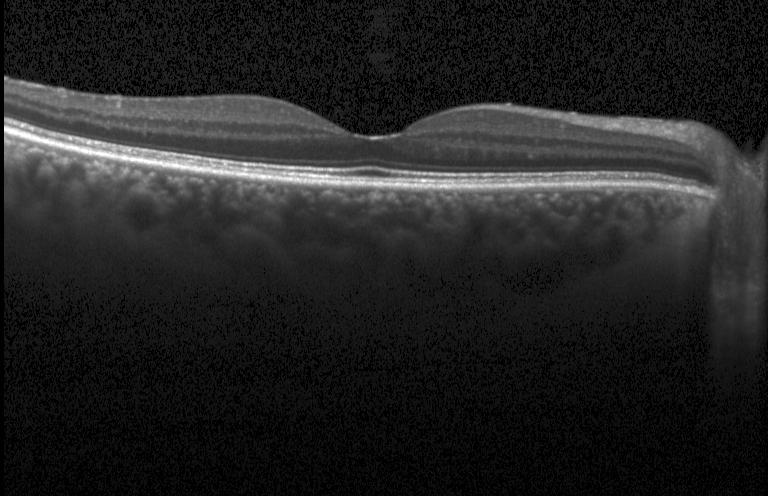

Optical coherence tomography B-scan. No choroidal neovascularization, diabetic macular edema, or drusen.